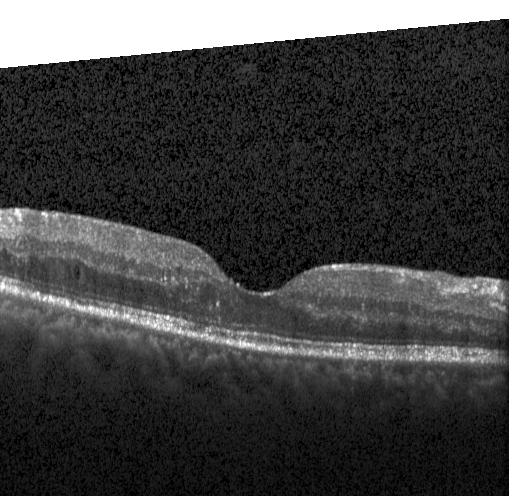
Impression: diabetic macular edema.